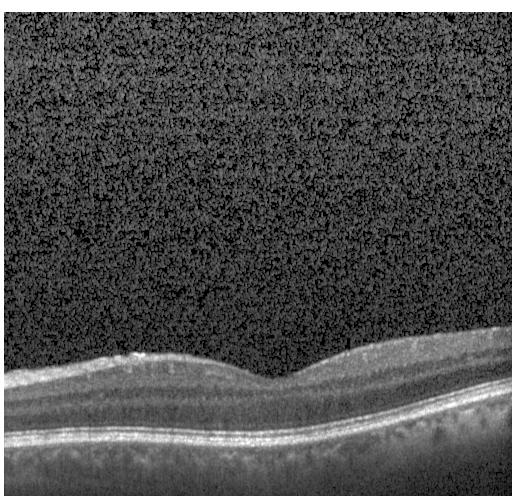 Retinal OCT B-scan. Fovea-centered. Neither CNV, DME, nor drusen.